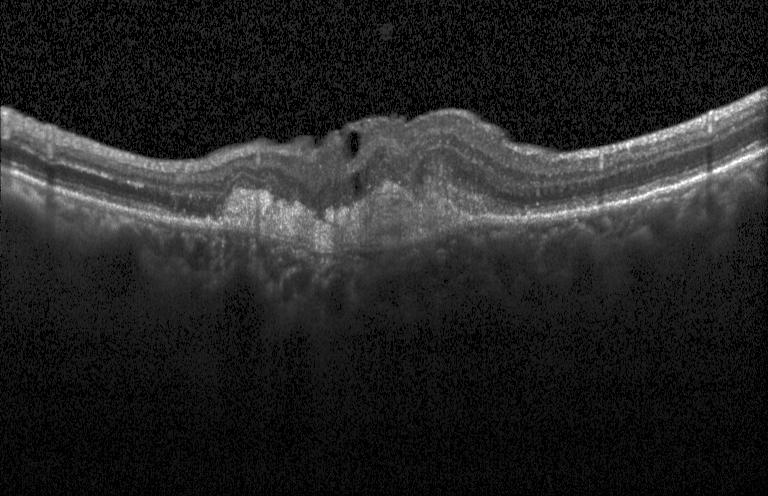
Impression: choroidal neovascularization.